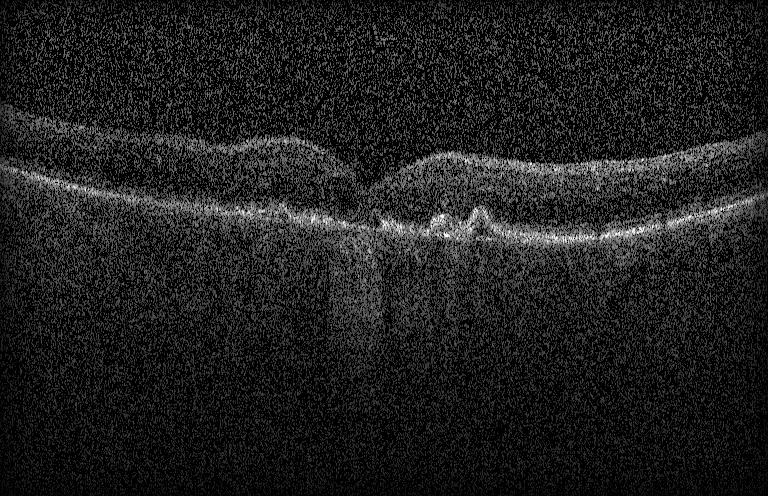
Optical coherence tomography B-scan, Heidelberg Spectralis — Diagnosis: a choroidal neovascular membrane.